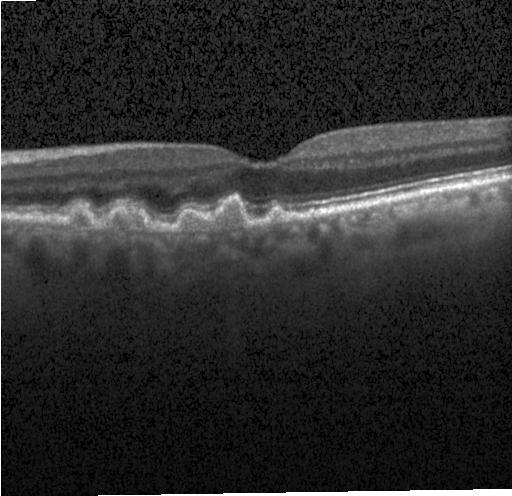

OCT line scan.
Assessment: sub-RPE drusenoid deposits.